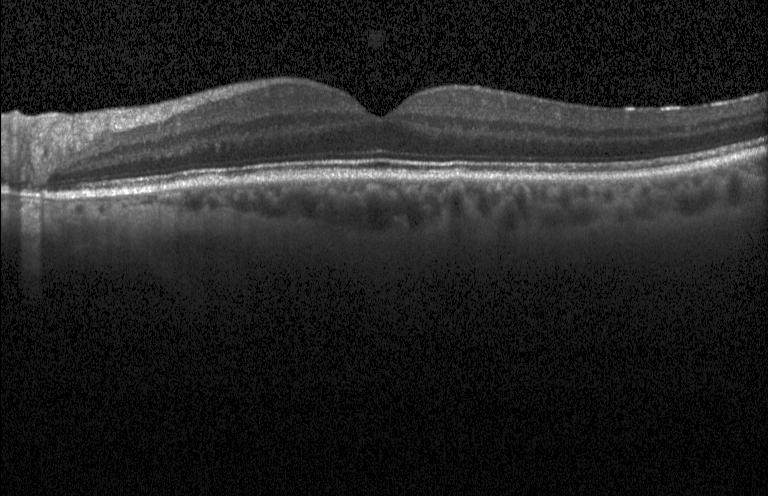
Optical coherence tomography B-scan — Finding: no evidence of choroidal neovascularization, diabetic macular edema, or drusen.